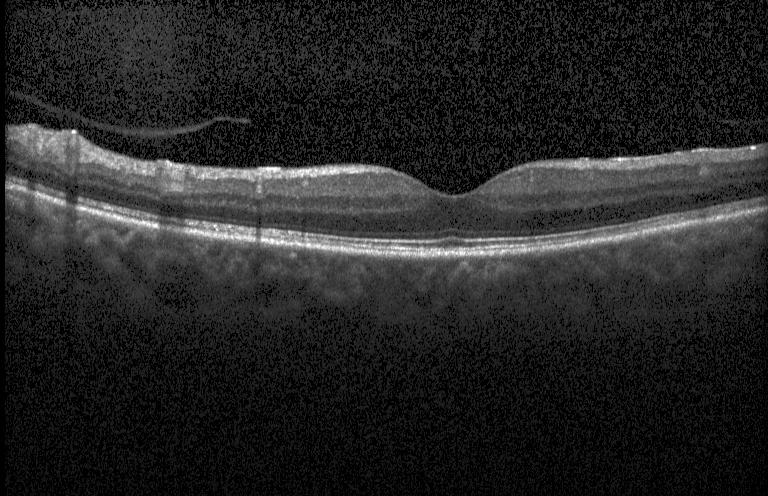 OCT line scan; fovea-centered.
This B-scan demonstrates no evidence of choroidal neovascularization, diabetic macular edema, or drusen.